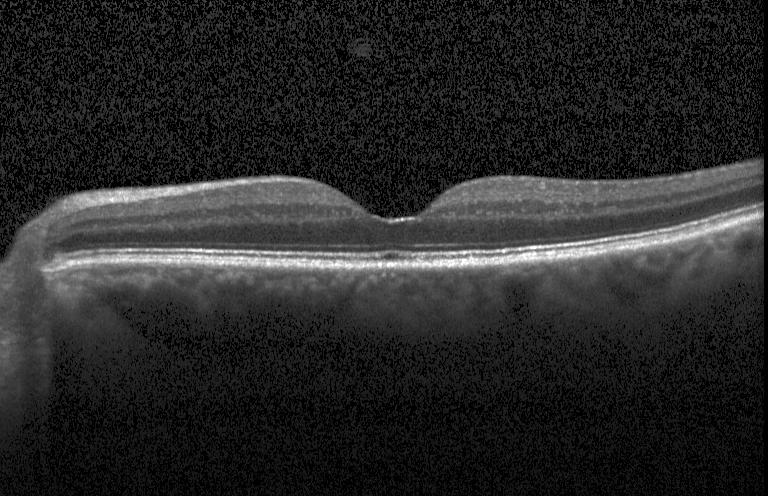 Horizontal scan through the fovea · retinal OCT cross-section · instrument: Heidelberg Spectralis · spectral-domain optical coherence tomography. Impression: no choroidal neovascularization, no diabetic macular edema, and no drusen.